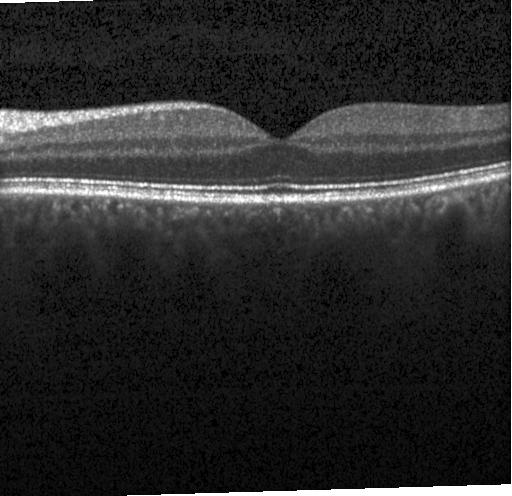
This B-scan demonstrates no evidence of choroidal neovascularization, diabetic macular edema, or drusen.